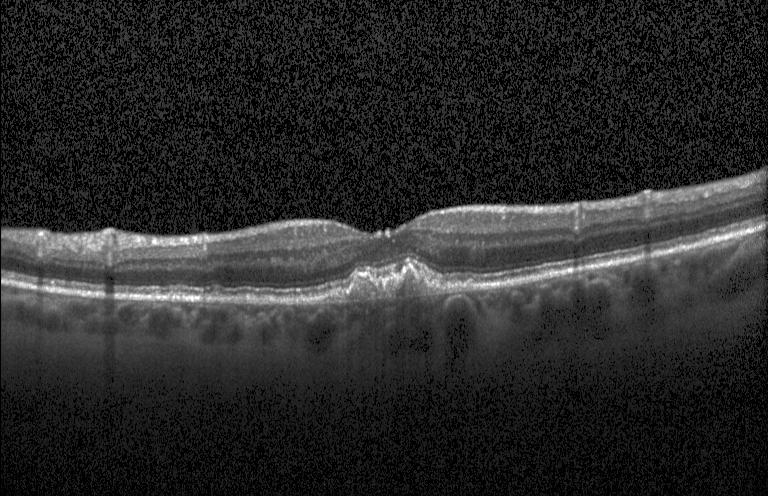
Diagnosis: multiple drusen.